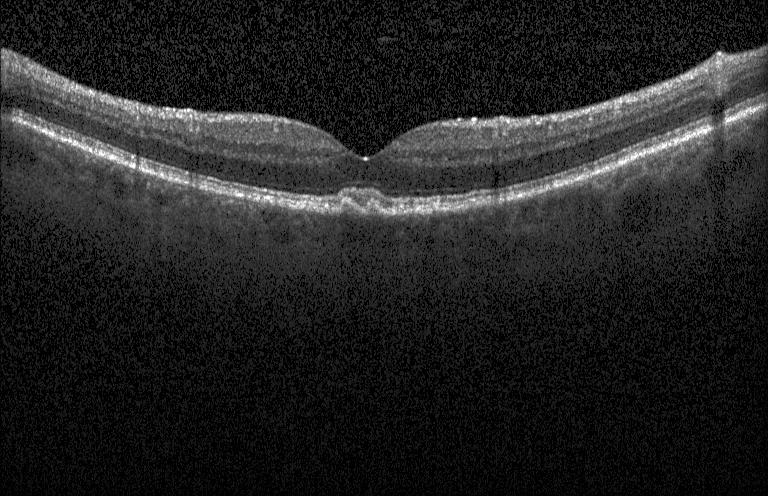

Retinal OCT cross-section
Diagnosis: sub-RPE drusenoid deposits.